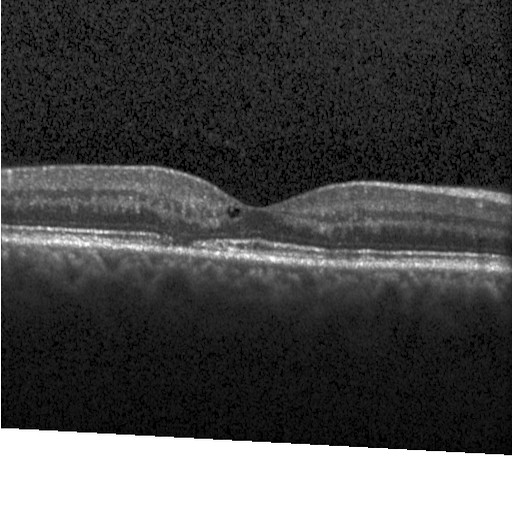

Diabetic macular edema (DME).